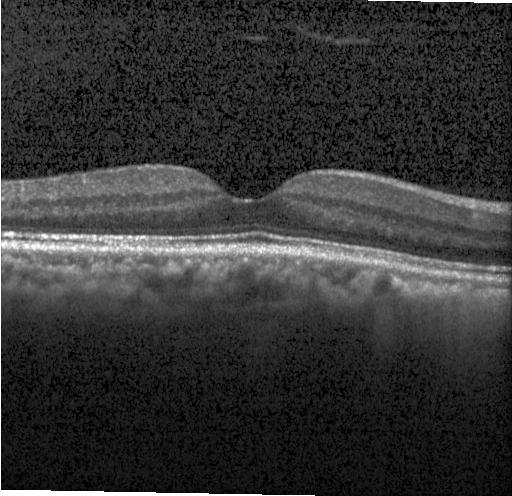 Spectral-domain optical coherence tomography. Horizontal scan through the fovea. OCT line scan — No choroidal neovascularization, no diabetic macular edema, and no drusen.